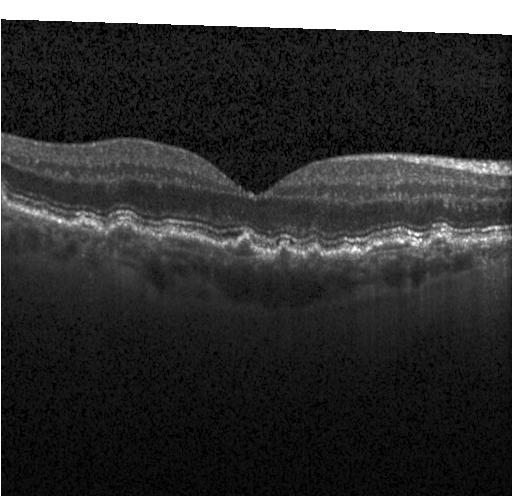

OCT B-scan; horizontal scan through the fovea — OCT finding: multiple drusen.